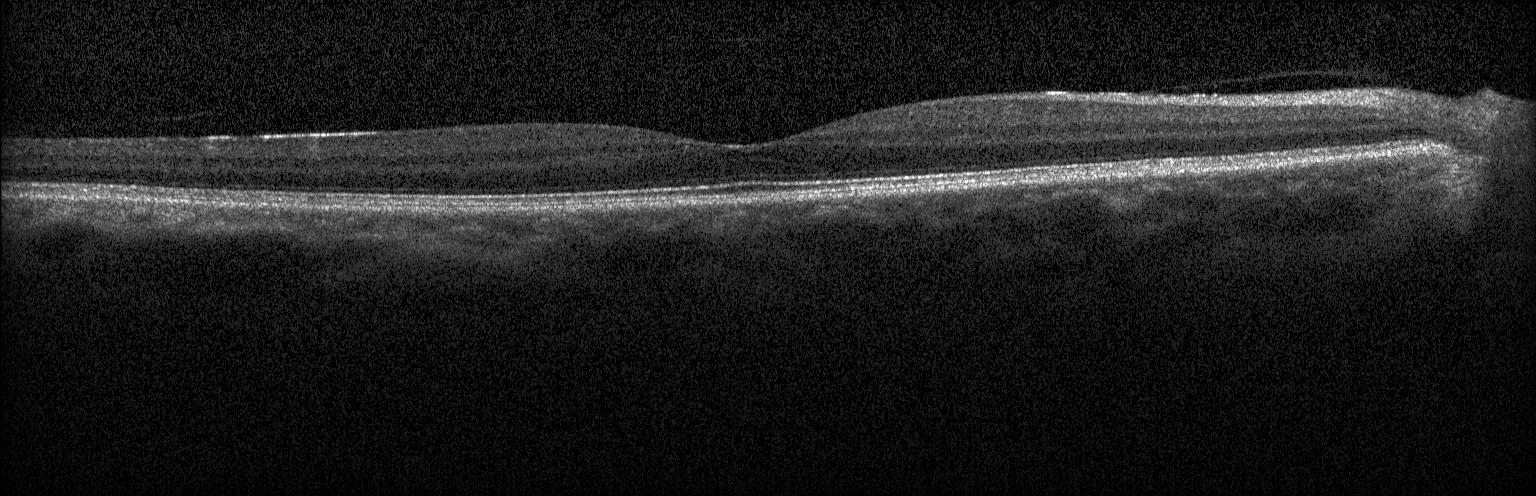

Diagnosis: no choroidal neovascularization, no diabetic macular edema, and no drusen.